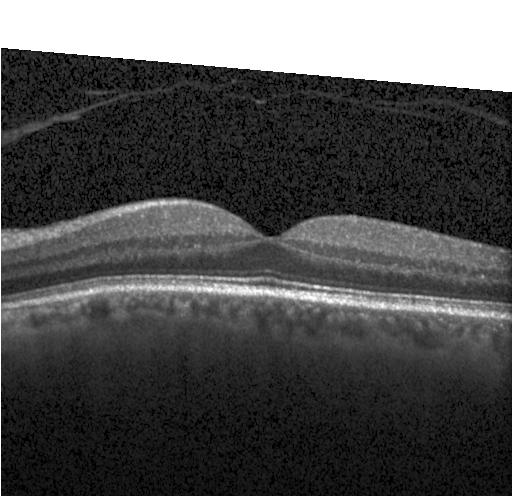 Finding: no evidence of choroidal neovascularization, diabetic macular edema, or drusen.